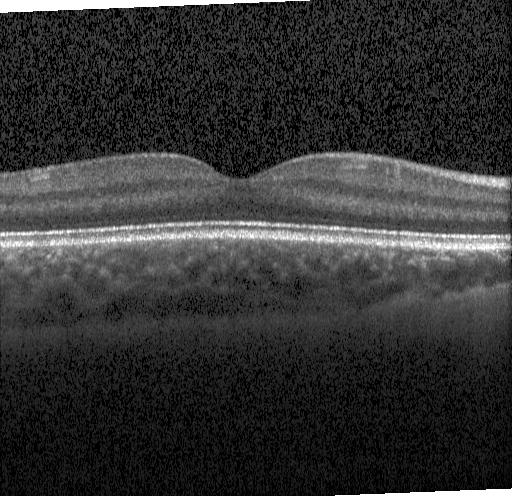 Centered on the fovea. SD-OCT. OCT line scan — Diagnosis: no evidence of choroidal neovascularization, diabetic macular edema, or drusen.